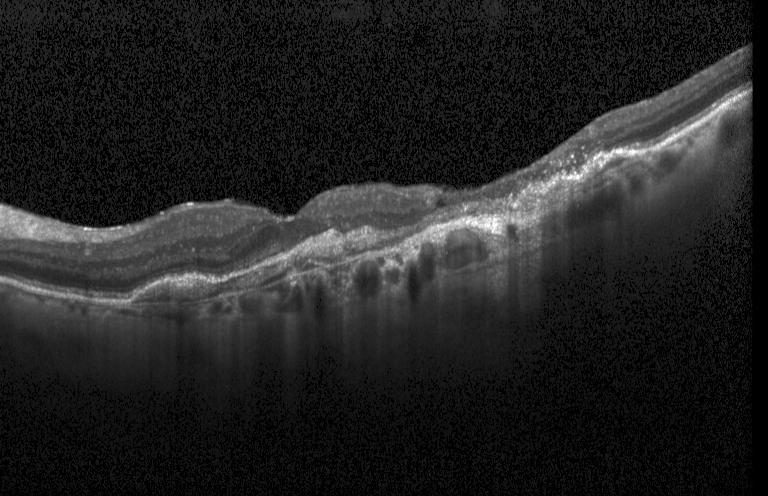
Optical coherence tomography B-scan. Heidelberg Spectralis OCT system. Through the macula. SD-OCT. Dx: choroidal neovascularization (CNV).